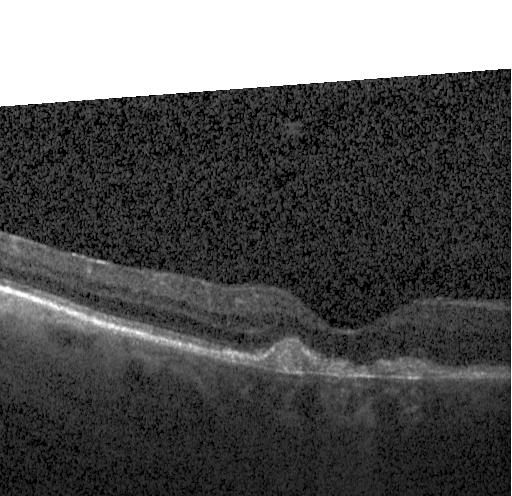

OCT B-scan.
The scan shows a choroidal neovascular membrane.